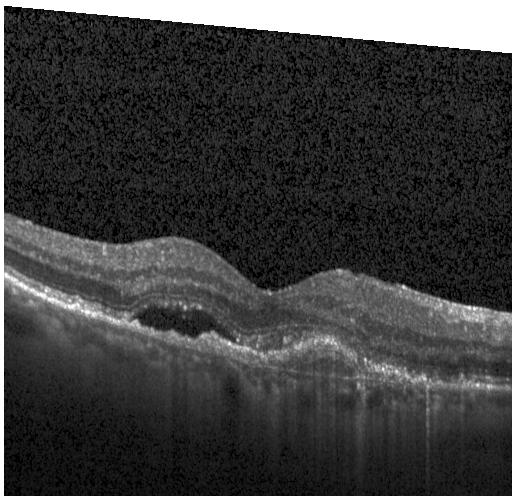
Impression: a choroidal neovascular membrane.